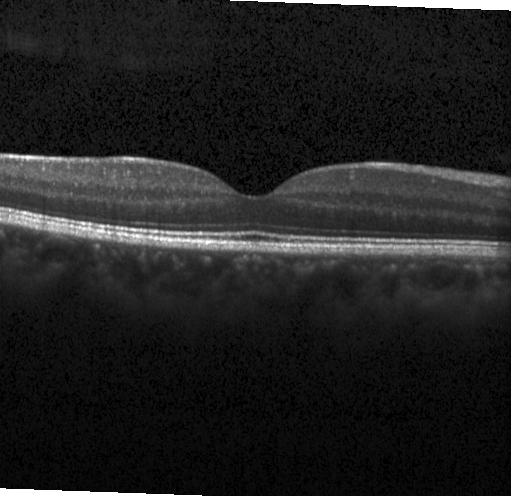

SD-OCT · macular scan · retinal OCT cross-section · acquired on a Heidelberg Spectralis.
Dx: no choroidal neovascularization, no diabetic macular edema, and no drusen.